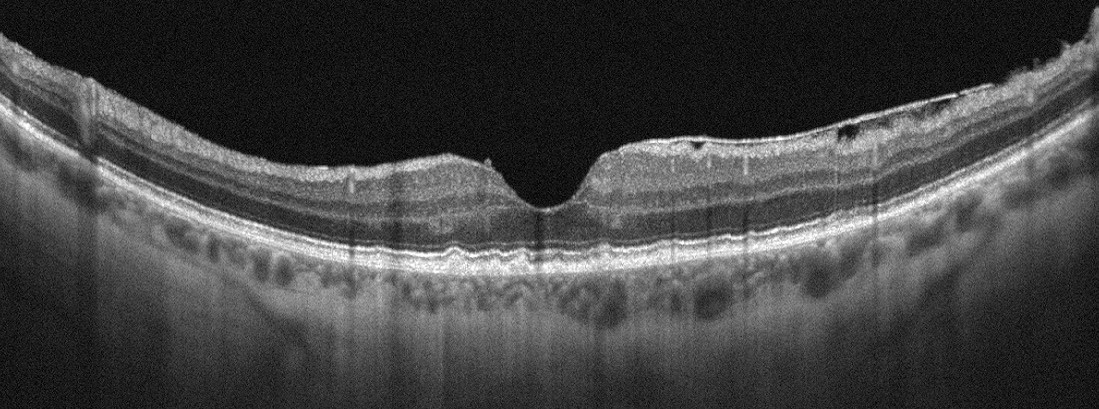 Diagnosis: AMD.